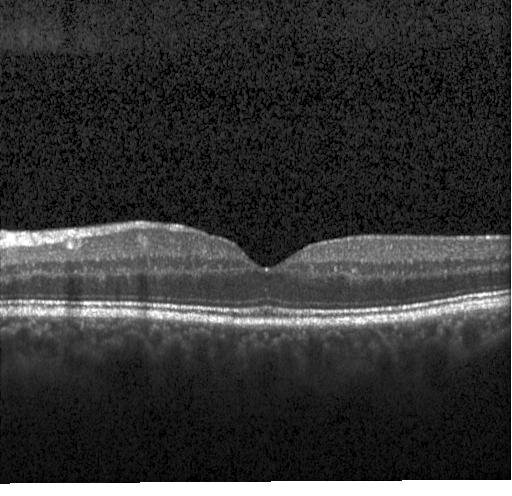 Heidelberg Spectralis OCT system, optical coherence tomography scan
Finding: no evidence of choroidal neovascularization, diabetic macular edema, or drusen.